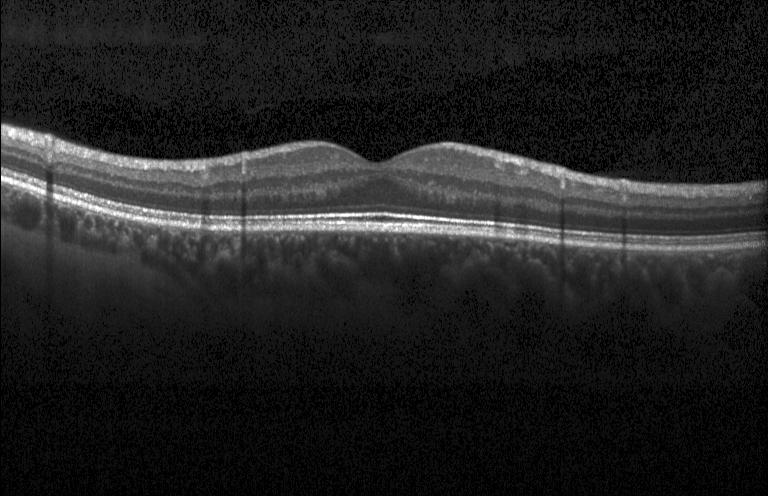 Dx: neither choroidal neovascularization, diabetic macular edema, nor drusen.